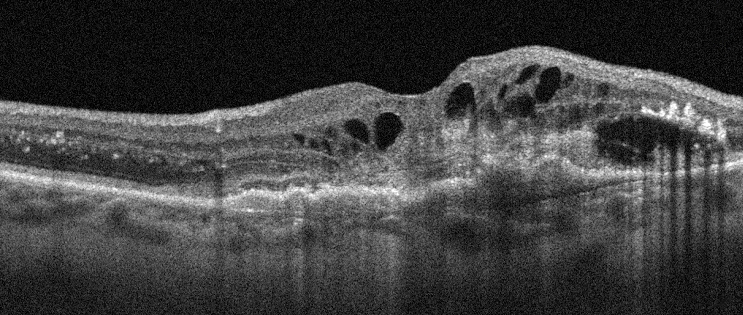

Retinal OCT cross-section — Diagnosis: age-related macular degeneration (AMD).